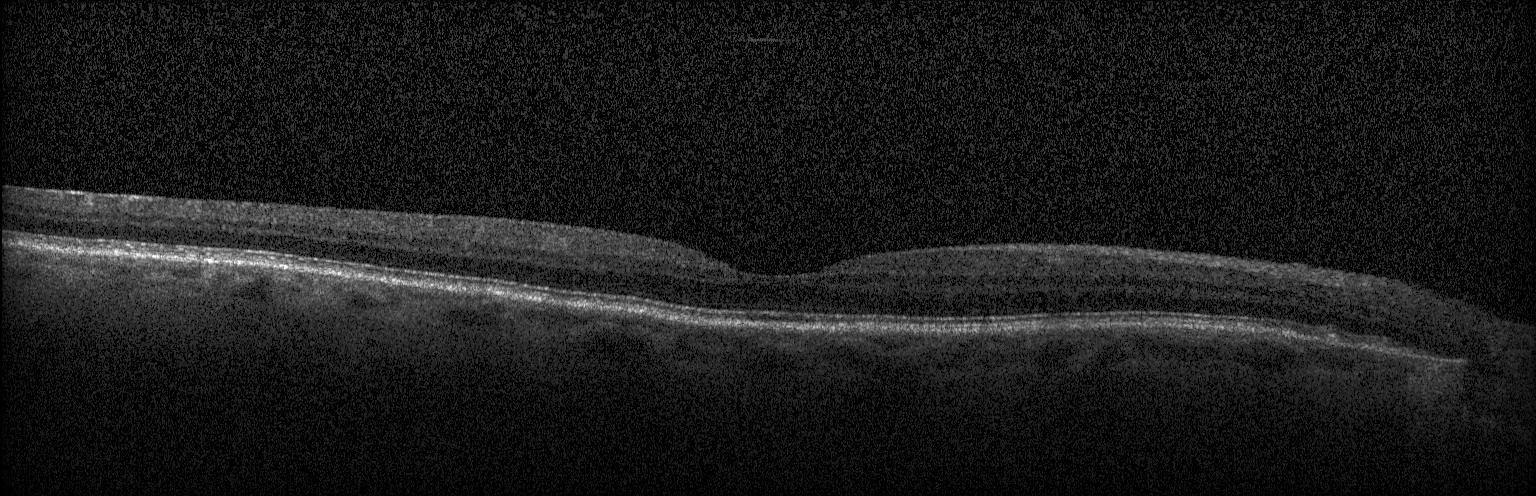

OCT finding: no choroidal neovascularization, no diabetic macular edema, and no drusen.